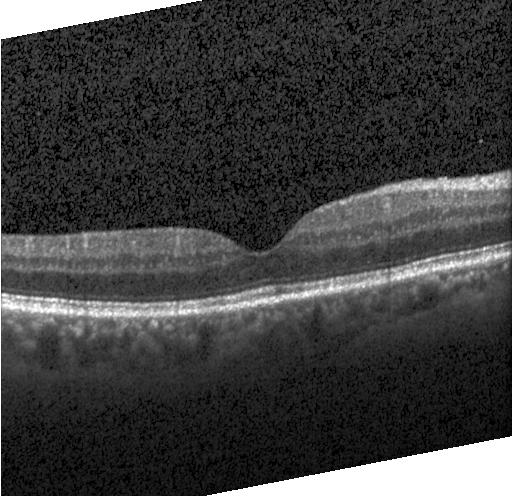

OCT B-scan; instrument: Heidelberg Spectralis; spectral-domain optical coherence tomography; horizontal scan through the fovea — OCT finding: neither CNV, DME, nor drusen.